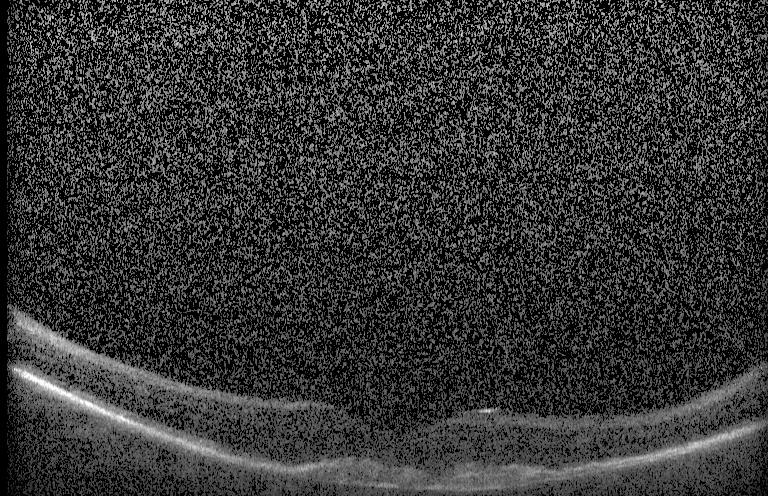 Retinal OCT cross-section. SD-OCT.
Dx: choroidal neovascularization (CNV).